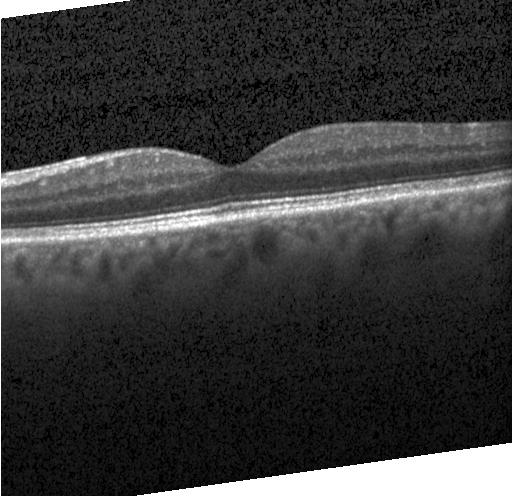 Diagnosis: no choroidal neovascularization, diabetic macular edema, or drusen.